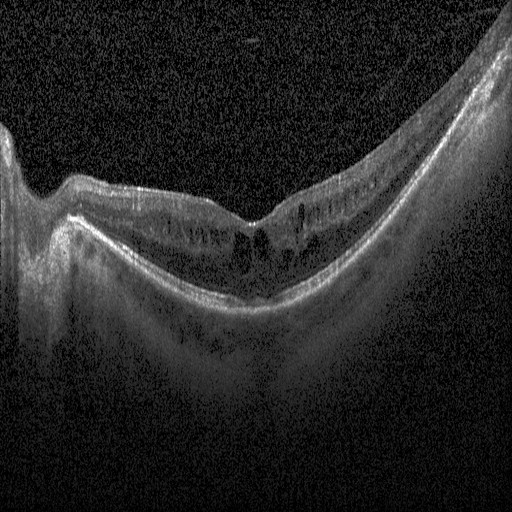

Finding: diabetic macular edema.